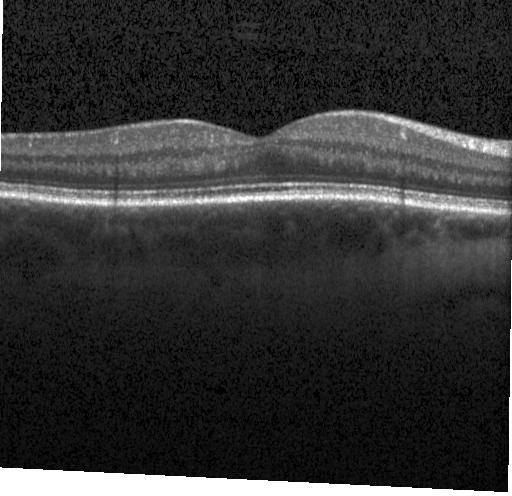
Heidelberg Spectralis OCT system. Retinal OCT cross-section. SD-OCT. This B-scan demonstrates no choroidal neovascularization, diabetic macular edema, or drusen.